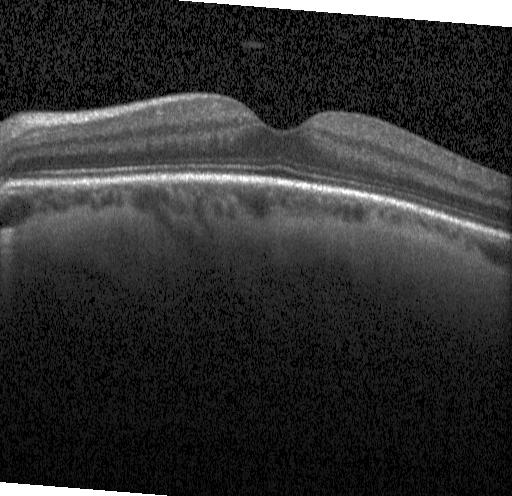
Heidelberg Spectralis OCT system · spectral-domain optical coherence tomography · through the macula · optical coherence tomography scan — OCT finding: no CNV, no DME, and no drusen.